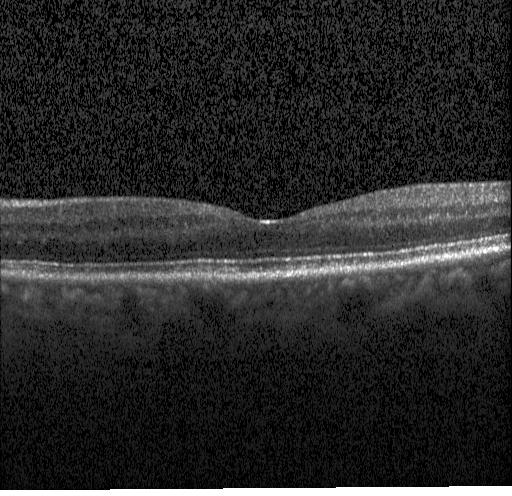
Acquired on a Heidelberg Spectralis · SD-OCT · OCT B-scan · horizontal scan through the fovea. This B-scan demonstrates neither choroidal neovascularization, diabetic macular edema, nor drusen.